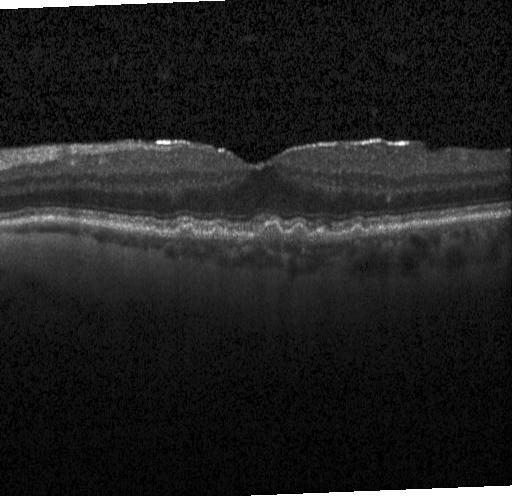
Diagnosis: multiple drusen.